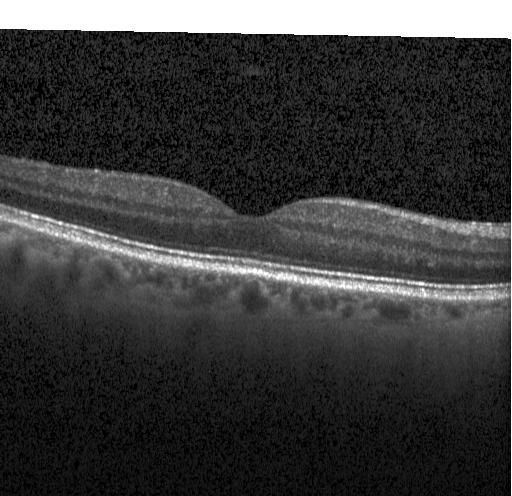

OCT finding: neither CNV, DME, nor drusen.